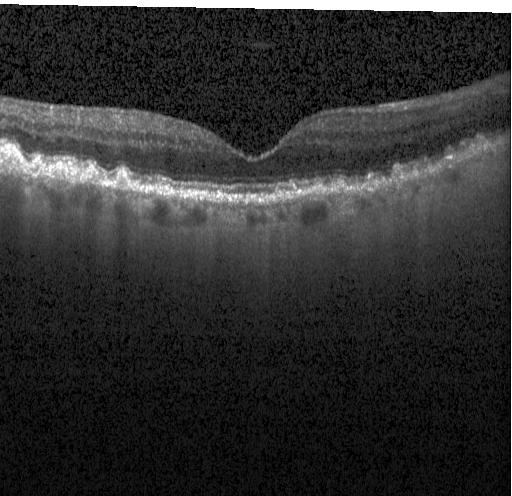

OCT B-scan
Diagnosis: sub-RPE drusenoid deposits.